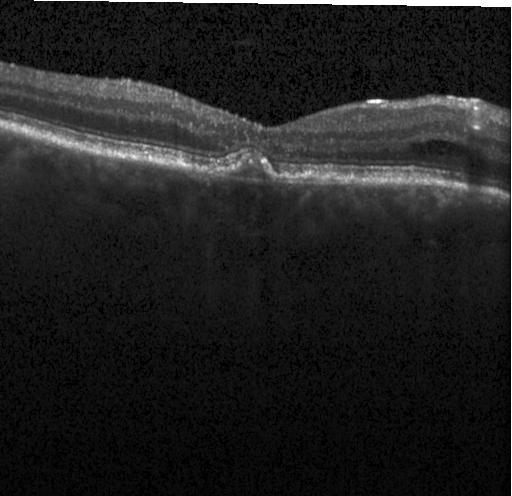

Finding: drusen.